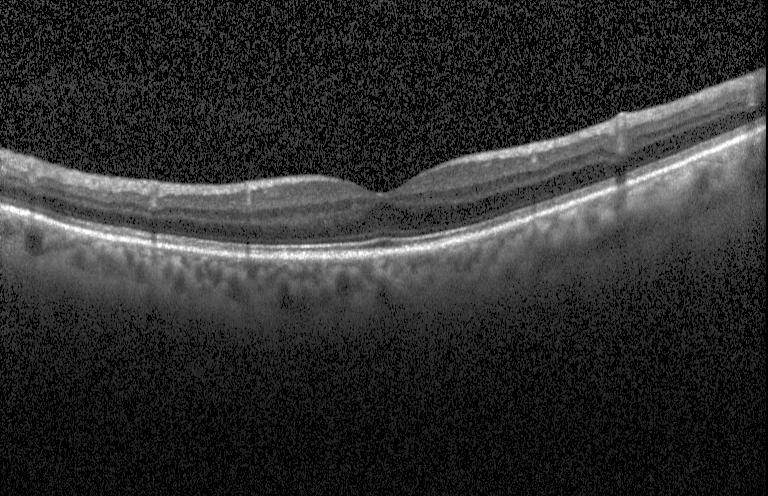
This B-scan demonstrates no choroidal neovascularization, diabetic macular edema, or drusen.